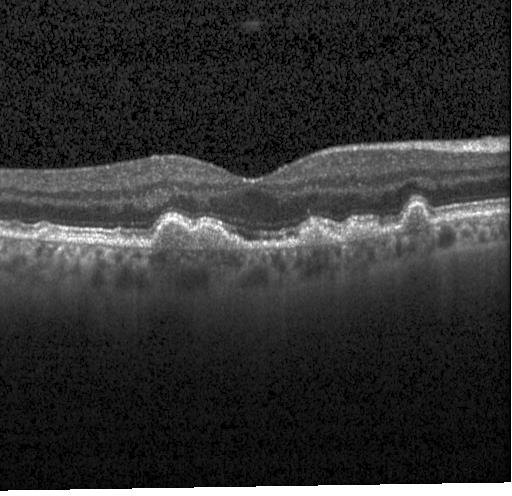 Impression: multiple drusen.